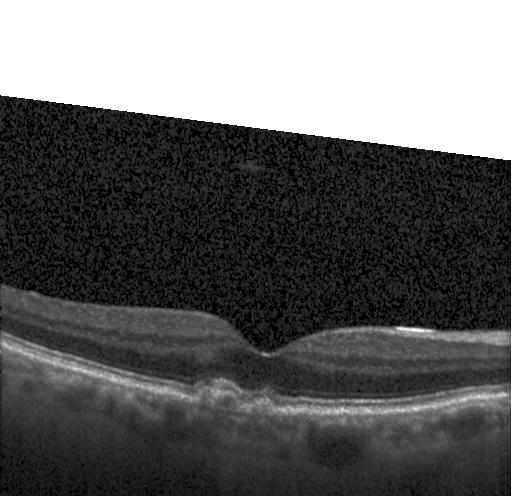
SD-OCT; retinal OCT cross-section; instrument: Heidelberg Spectralis; through the macula.
Finding: a choroidal neovascular membrane.